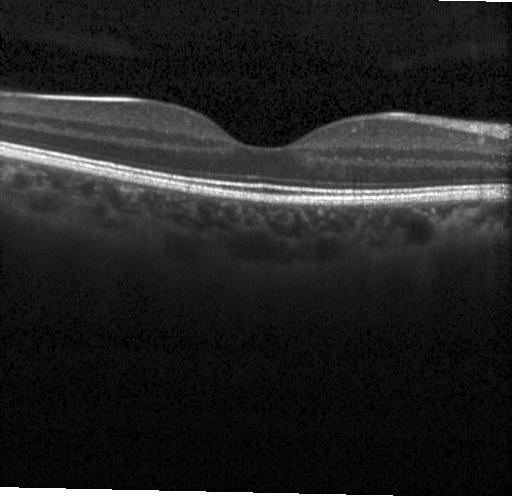

Finding: no choroidal neovascularization, no diabetic macular edema, and no drusen.